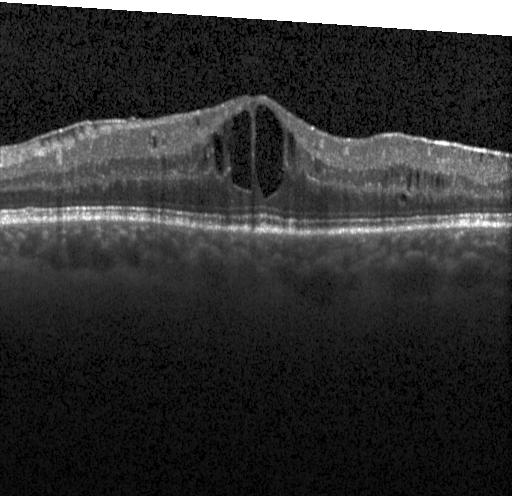
Heidelberg Spectralis, optical coherence tomography B-scan. This B-scan demonstrates diabetic macular edema.